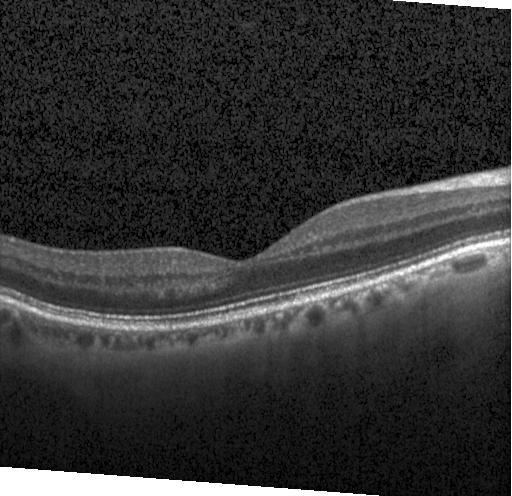

Centered on the fovea · OCT B-scan · SD-OCT — Finding: no CNV, no DME, and no drusen.